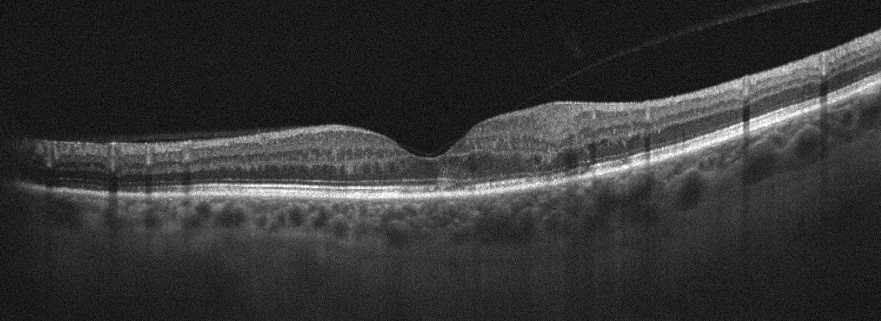

The scan shows diabetic macular edema.